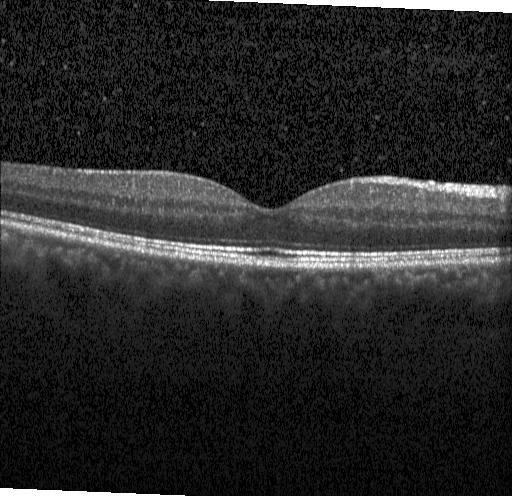
OCT line scan. SD-OCT. Horizontal scan through the fovea. Instrument: Heidelberg Spectralis — Impression: no evidence of choroidal neovascularization, diabetic macular edema, or drusen.